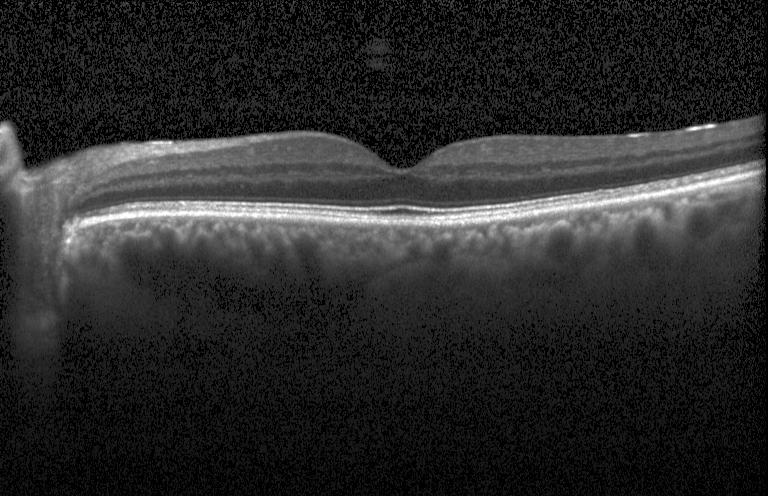 Optical coherence tomography B-scan; Heidelberg Spectralis — OCT finding: no evidence of CNV, DME, or drusen.